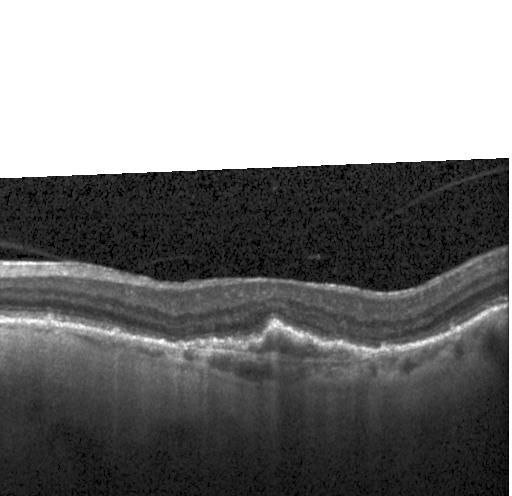 Spectral-domain OCT. Optical coherence tomography B-scan — Diagnosis: CNV.